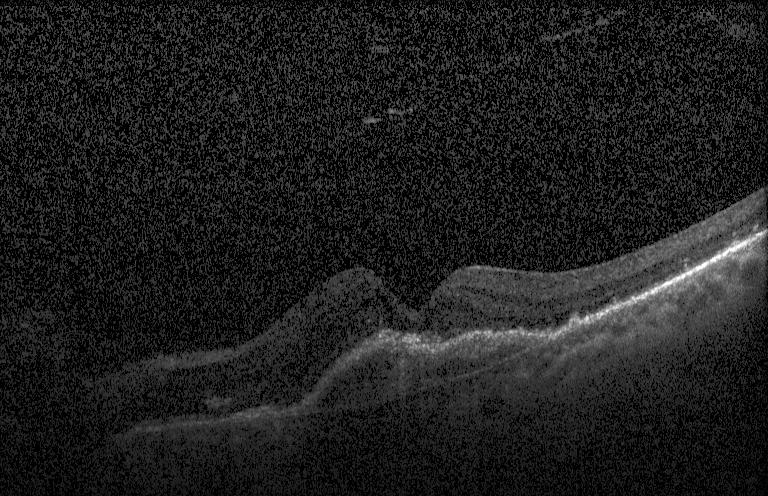
Macular scan. OCT B-scan. Heidelberg Spectralis. Spectral-domain OCT — Impression: a choroidal neovascular membrane.